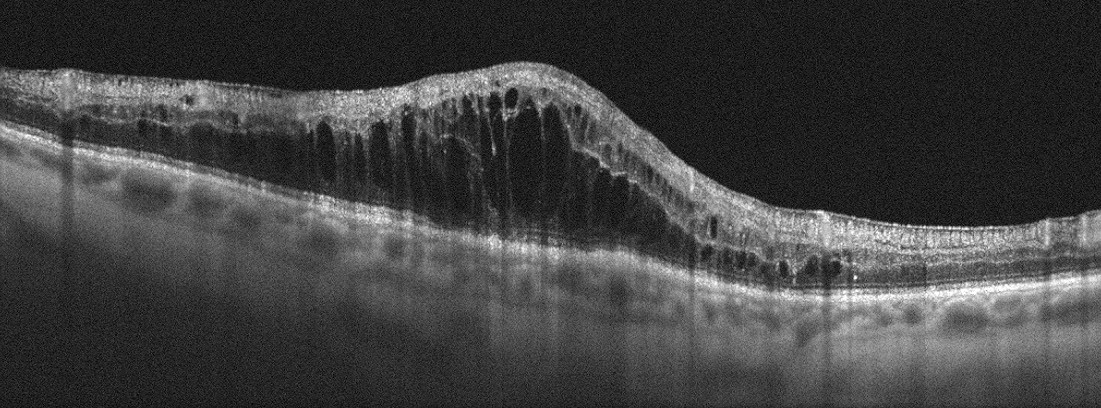

Retinal OCT B-scan — Dx: retinal vein occlusion.